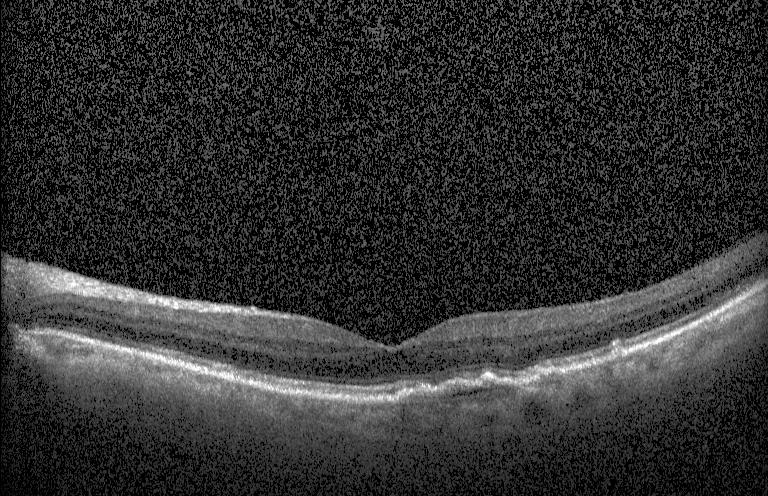
Acquired on a Heidelberg Spectralis, retinal OCT B-scan
This B-scan demonstrates choroidal neovascularization.